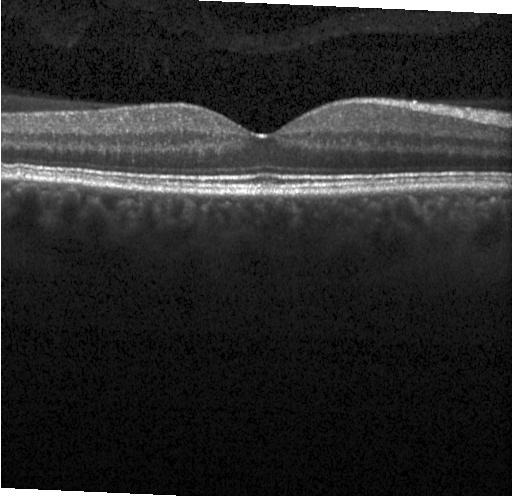
Optical coherence tomography scan
Impression: neither CNV, DME, nor drusen.